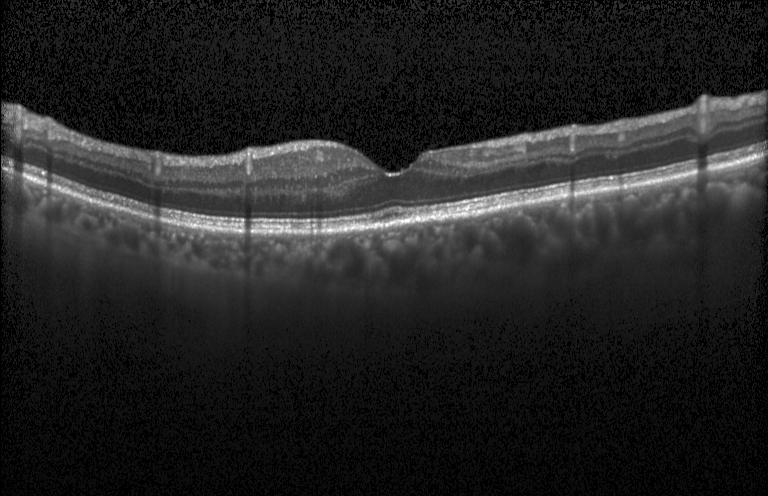

Instrument: Heidelberg Spectralis; optical coherence tomography scan; centered on the fovea; SD-OCT
Neither choroidal neovascularization, diabetic macular edema, nor drusen.